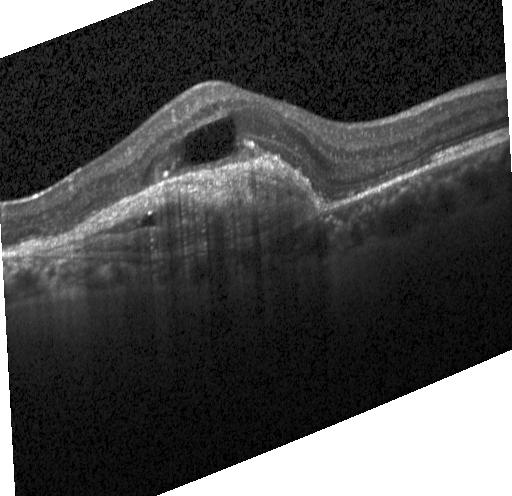
Horizontal scan through the fovea. Heidelberg Spectralis. Optical coherence tomography scan. Spectral-domain OCT — OCT finding: a choroidal neovascular membrane.